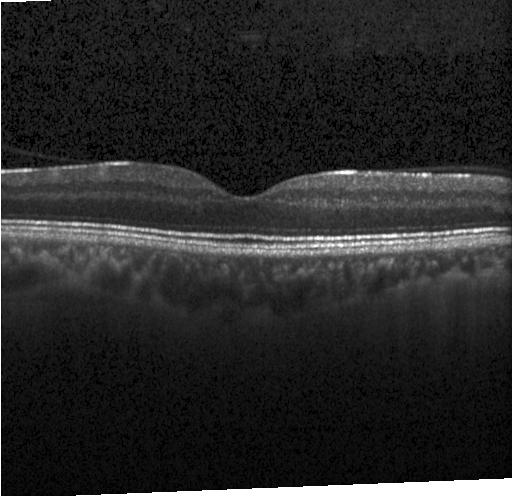

Optical coherence tomography scan, instrument: Heidelberg Spectralis, spectral-domain optical coherence tomography — Impression: no choroidal neovascularization, no diabetic macular edema, and no drusen.